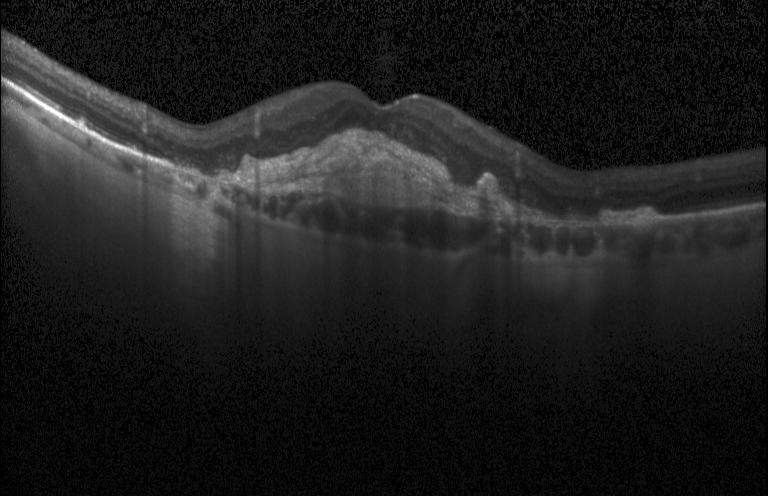
This B-scan demonstrates a choroidal neovascular membrane.